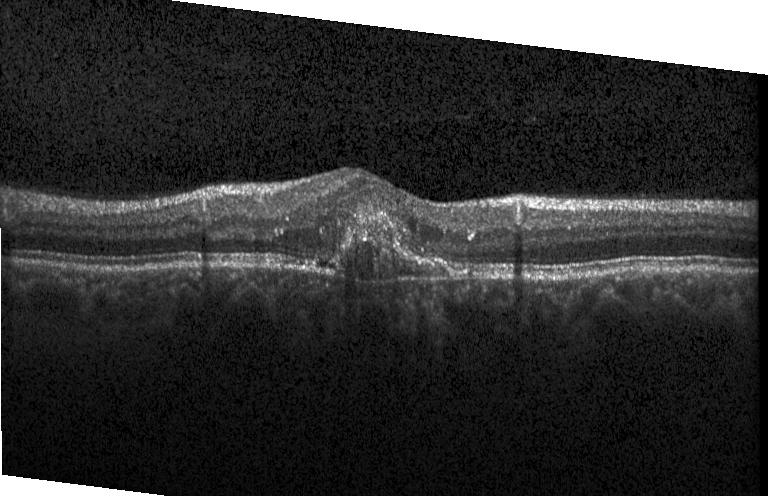 OCT B-scan showing choroidal neovascularization (CNV).